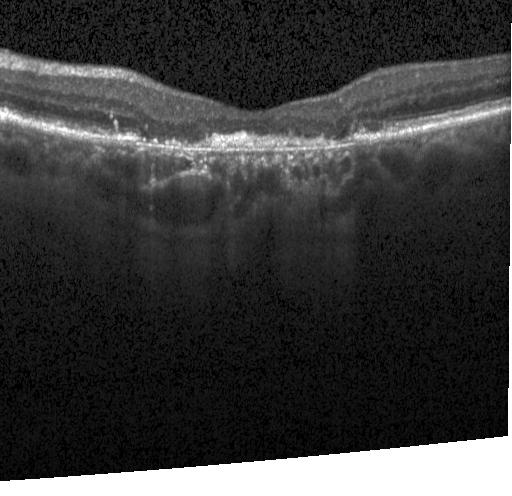

Finding: choroidal neovascularization (CNV).